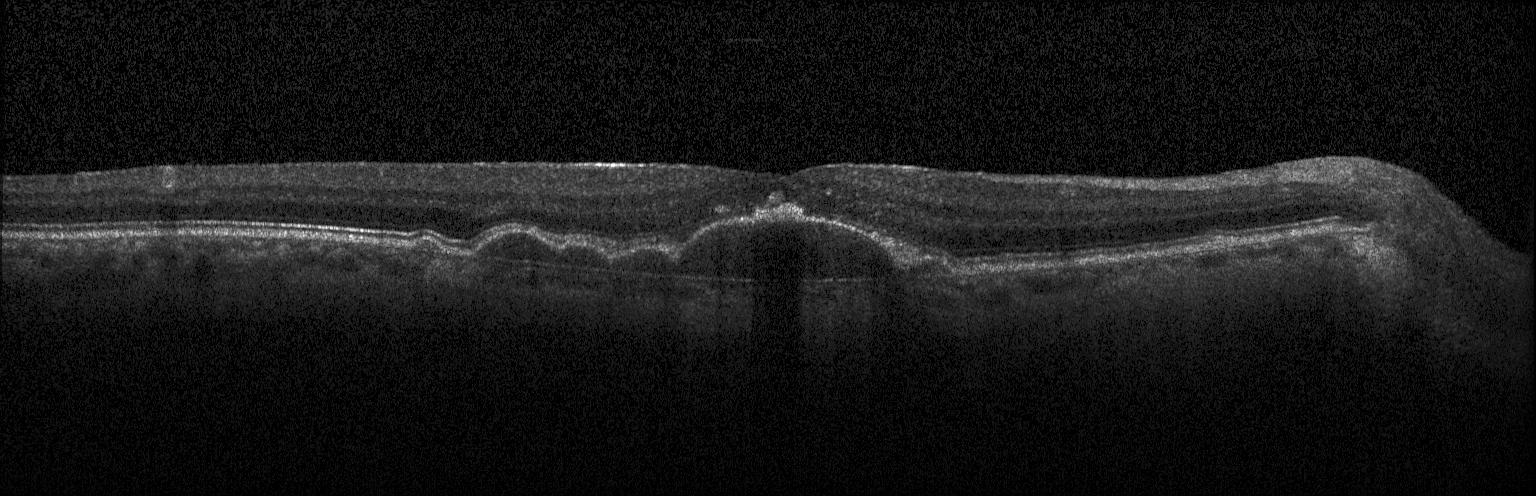

This B-scan demonstrates CNV.